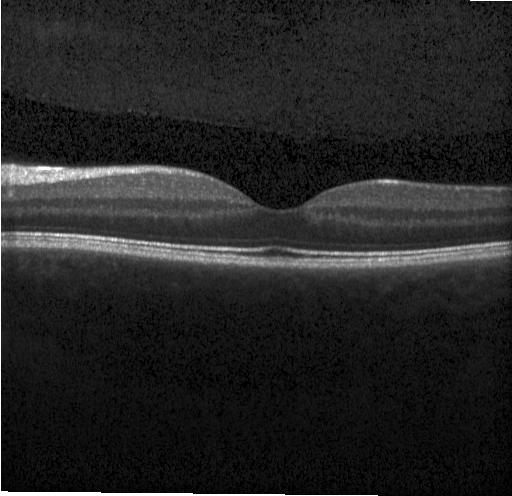

Spectral-domain optical coherence tomography. Retinal OCT B-scan — OCT finding: no evidence of CNV, DME, or drusen.